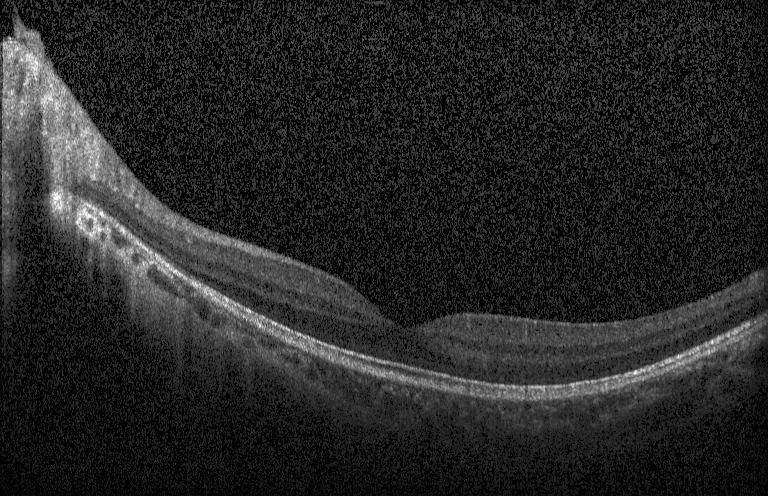
Diagnosis: no evidence of choroidal neovascularization, diabetic macular edema, or drusen.